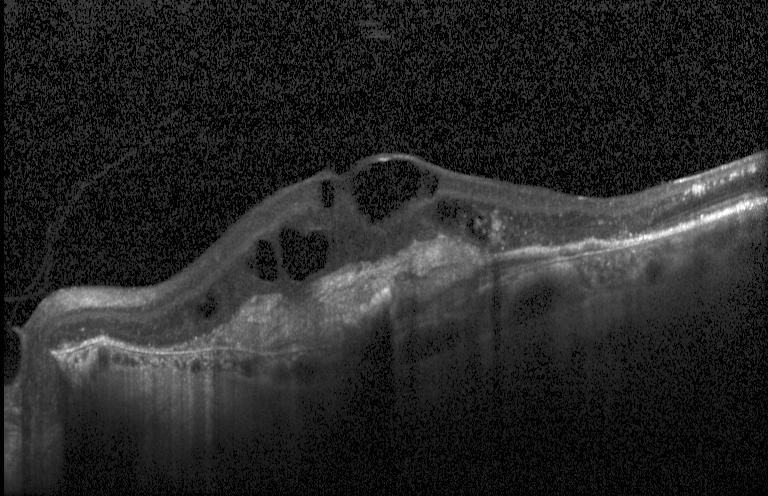 OCT B-scan.
Macular OCT: choroidal neovascularization (CNV).